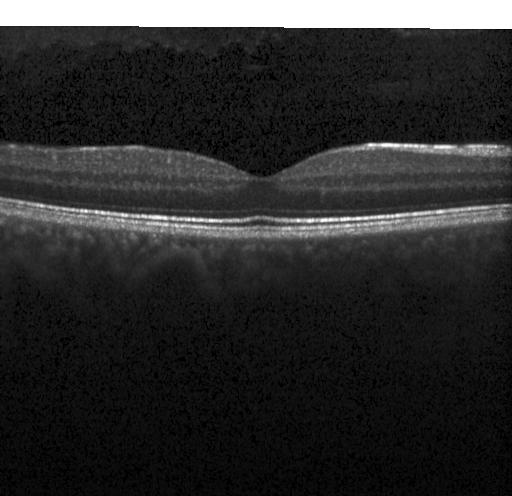 Optical coherence tomography scan. Finding: neither CNV, DME, nor drusen.